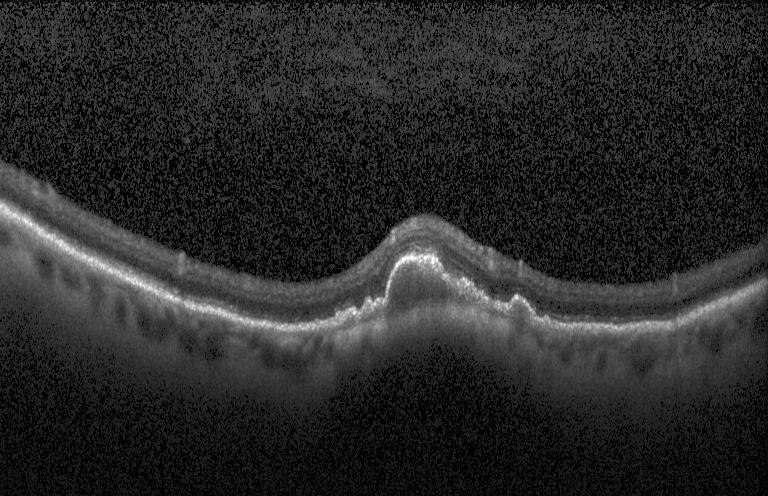
Retinal OCT B-scan — The scan shows a choroidal neovascular membrane.